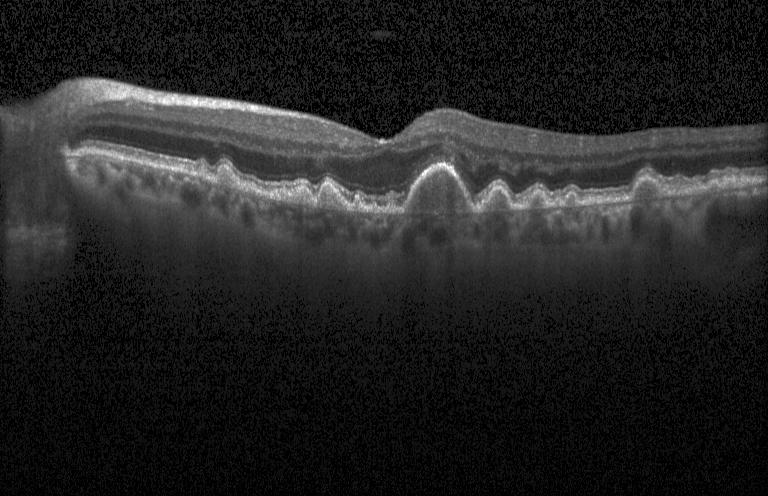

Dx: multiple drusen.